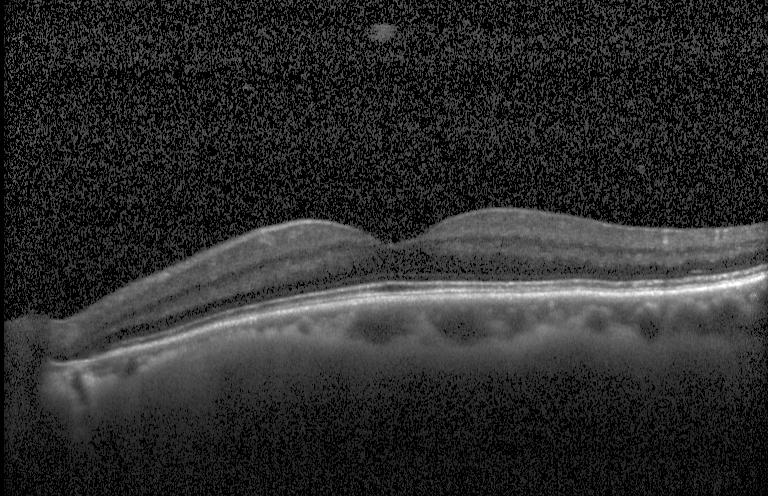

OCT line scan.
OCT finding: neither choroidal neovascularization, diabetic macular edema, nor drusen.